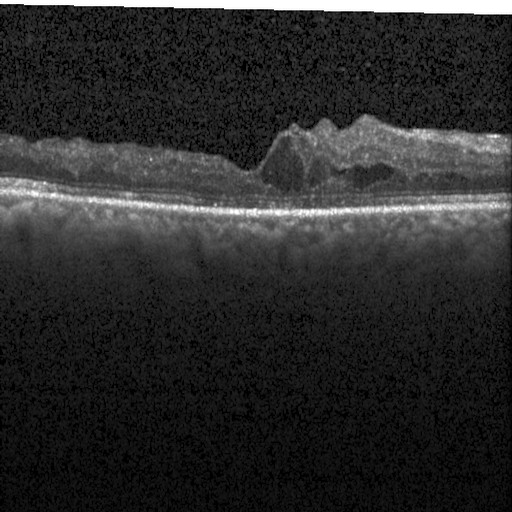

Impression: diabetic macular edema (DME).